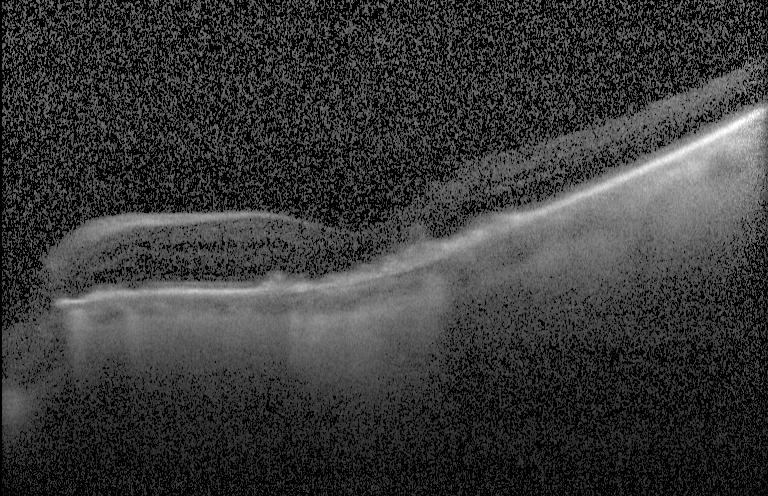

Spectral-domain OCT B-scan: a choroidal neovascular membrane.